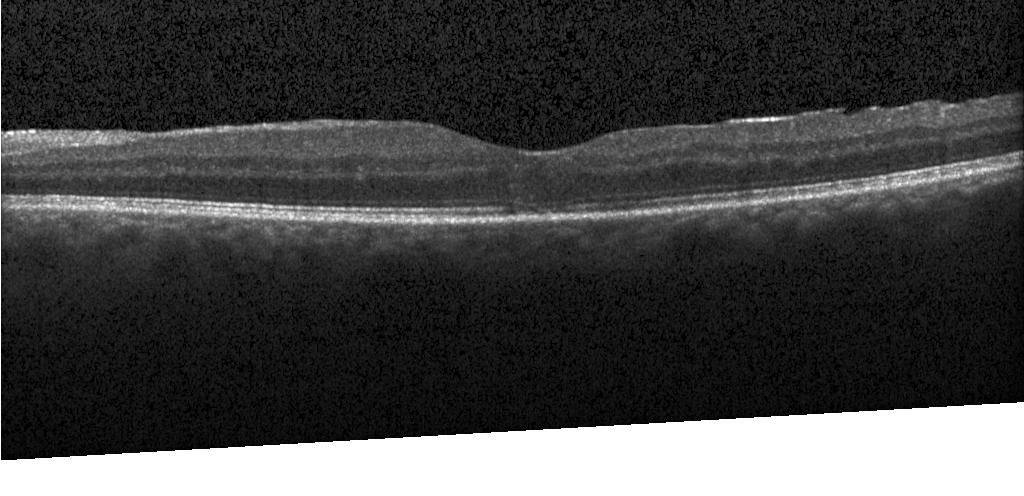

Centered on the fovea; optical coherence tomography scan; spectral-domain OCT; Heidelberg Spectralis — Finding: neither choroidal neovascularization, diabetic macular edema, nor drusen.